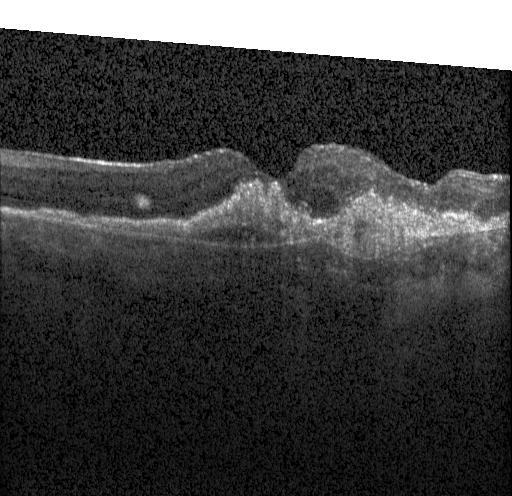

Horizontal scan through the fovea. Retinal OCT B-scan. Heidelberg Spectralis. Spectral-domain optical coherence tomography
OCT finding: a choroidal neovascular membrane.